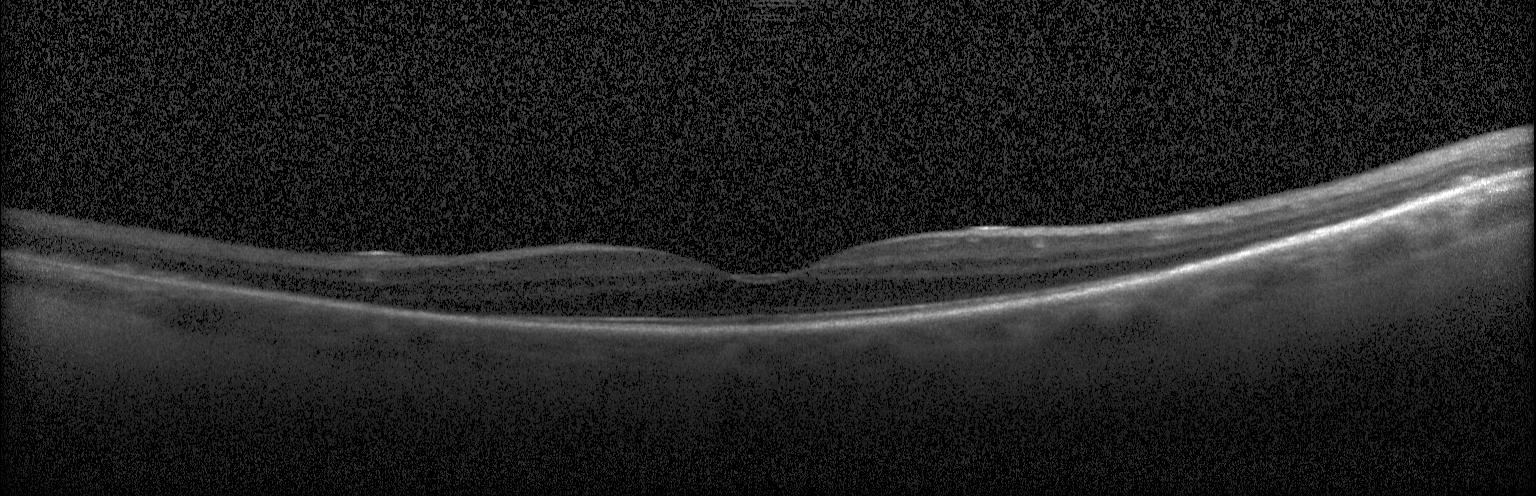 Optical coherence tomography B-scan. Through the macula. Spectral-domain OCT. The scan shows no evidence of choroidal neovascularization, diabetic macular edema, or drusen.